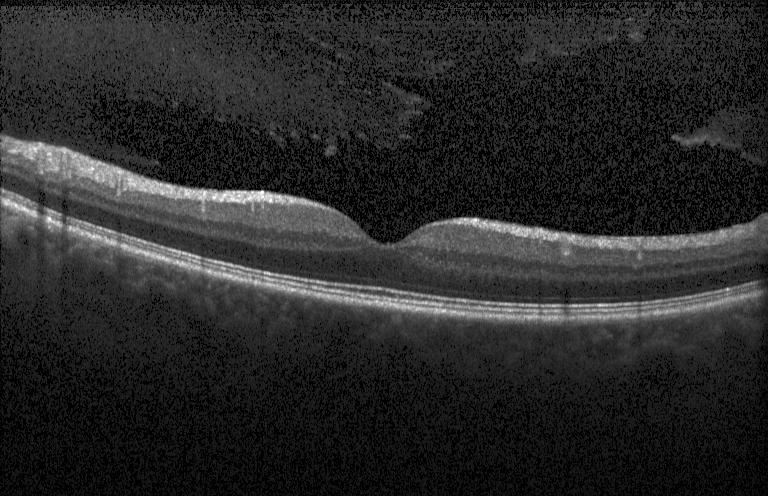
Impression: no CNV, no DME, and no drusen.